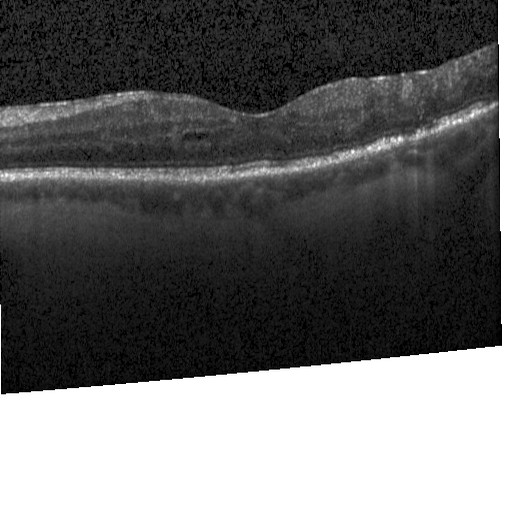

Assessment: diabetic macular edema.